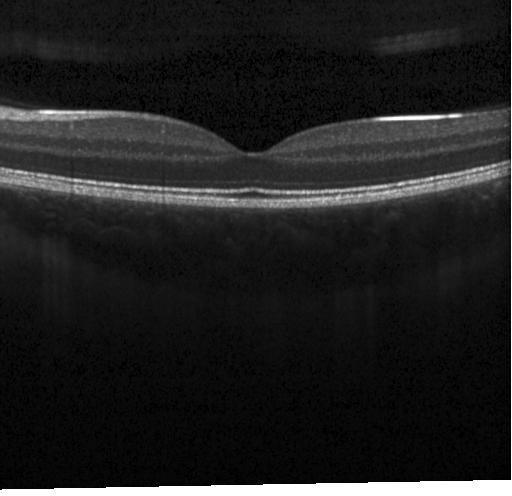
Retinal OCT B-scan · fovea-centered
Impression: no evidence of CNV, DME, or drusen.